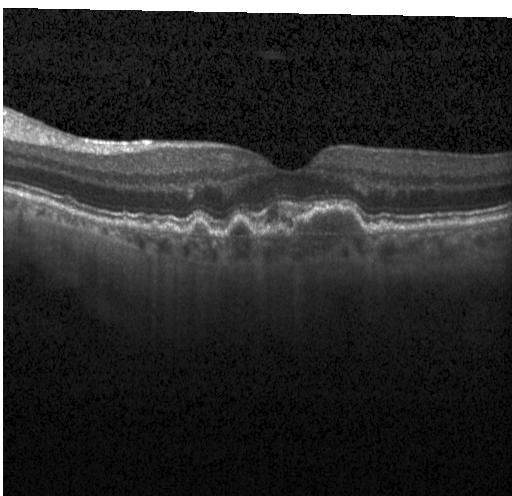
OCT scan showing drusen.